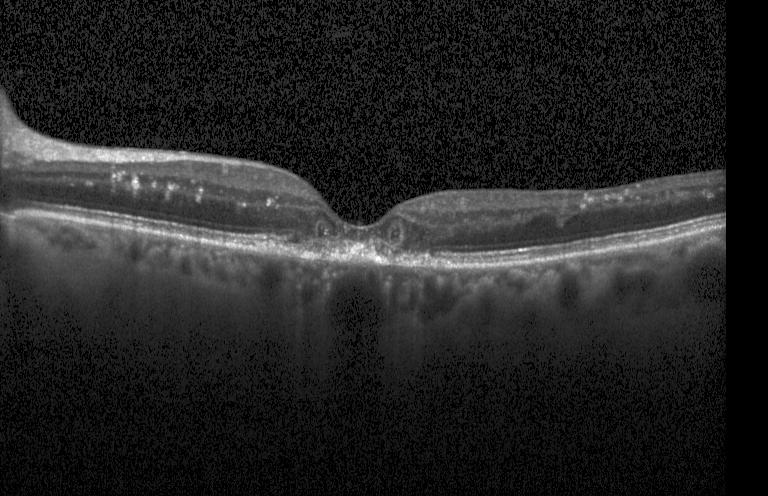 Centered on the fovea. OCT B-scan — Finding: a choroidal neovascular membrane.